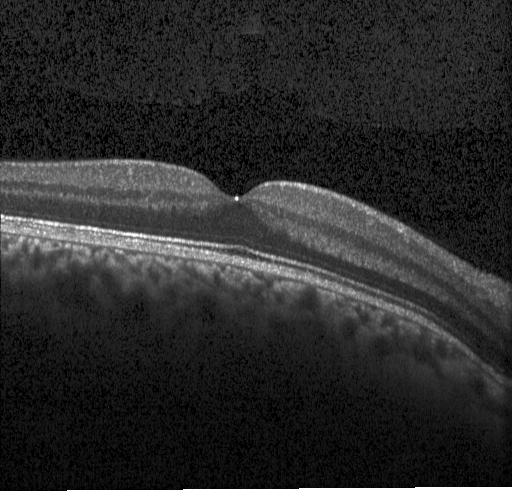
OCT B-scan.
Assessment: no CNV, DME, or drusen.